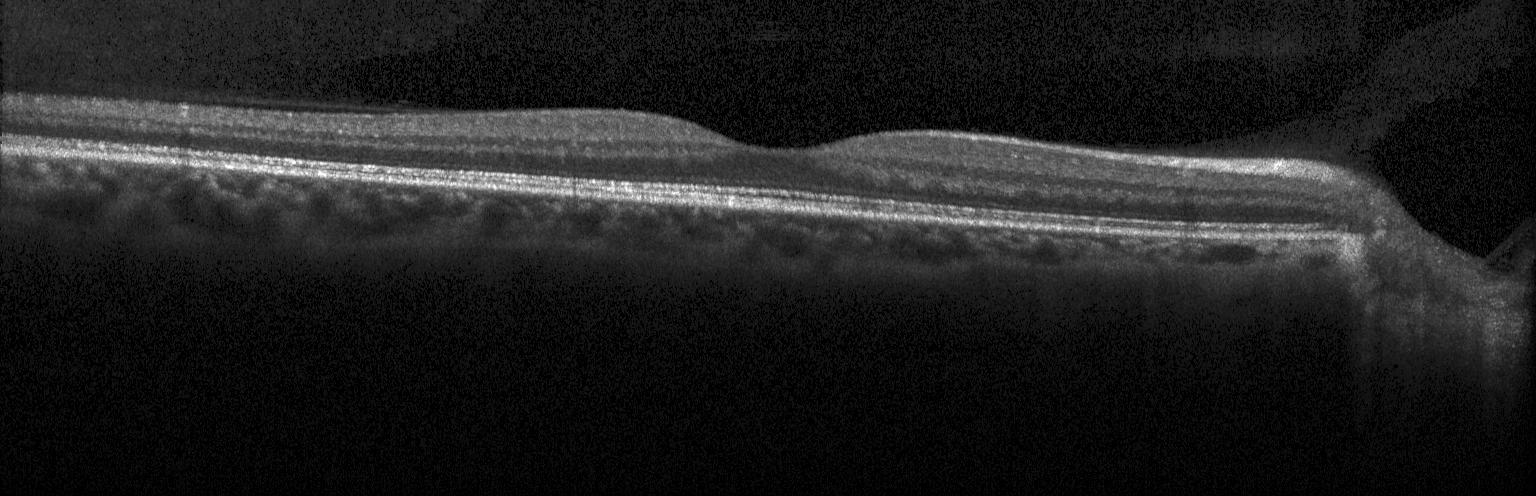
OCT finding: neither CNV, DME, nor drusen.